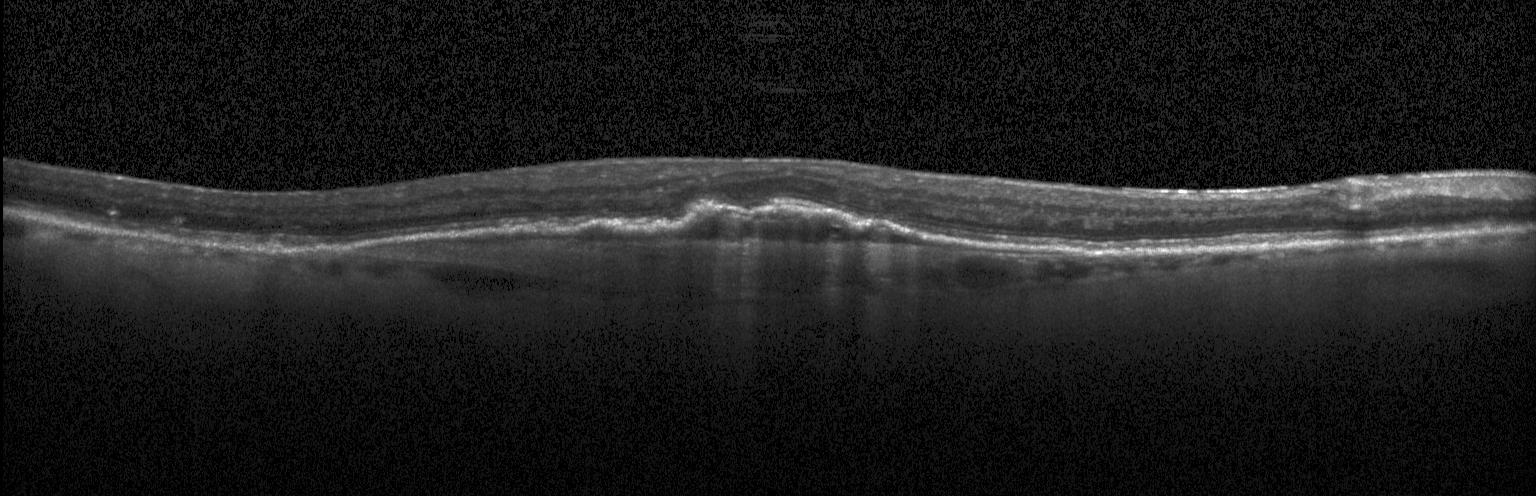

OCT finding: a choroidal neovascular membrane.